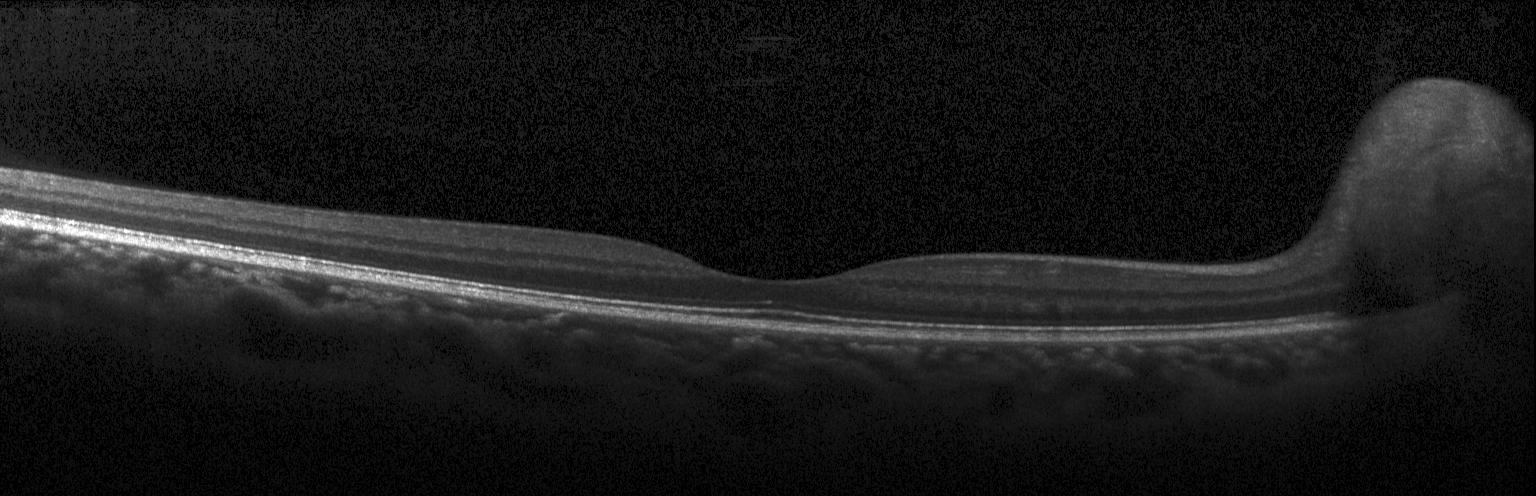 Assessment: no choroidal neovascularization, no diabetic macular edema, and no drusen.